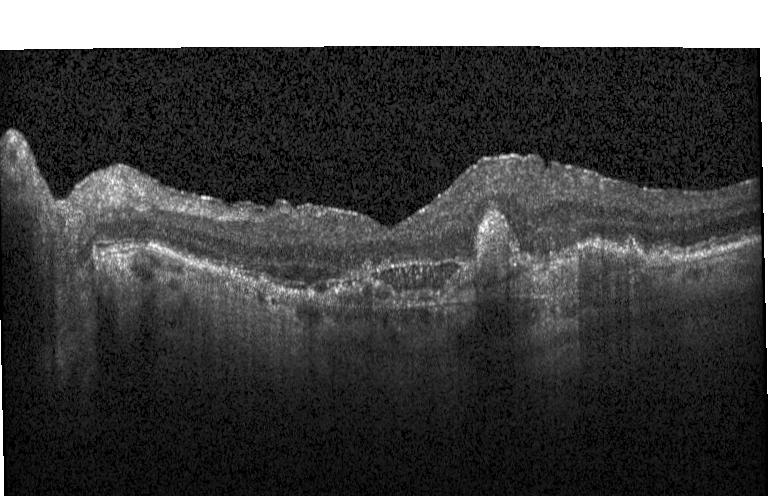 Spectral-domain optical coherence tomography. Optical coherence tomography B-scan.
CNV.